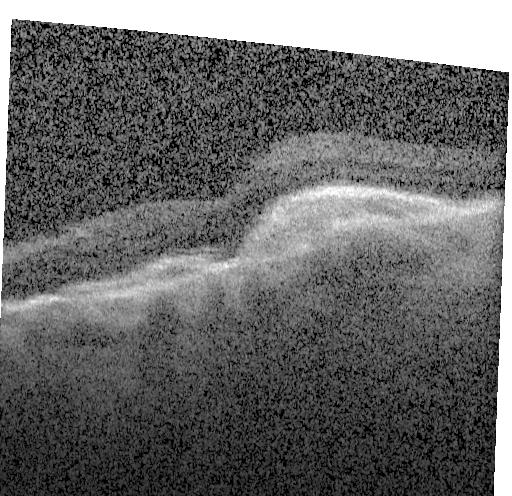 Finding: a choroidal neovascular membrane.